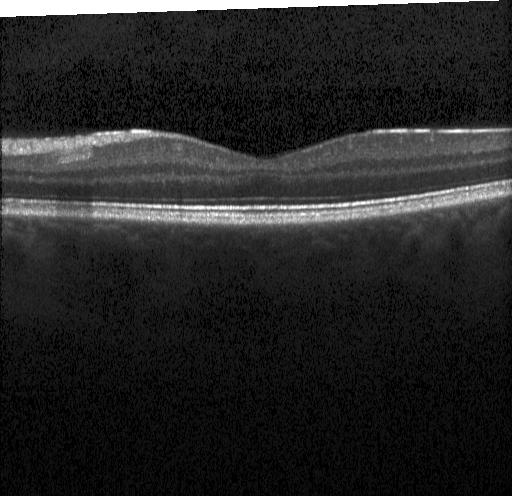
Optical coherence tomography scan — Dx: neither choroidal neovascularization, diabetic macular edema, nor drusen.